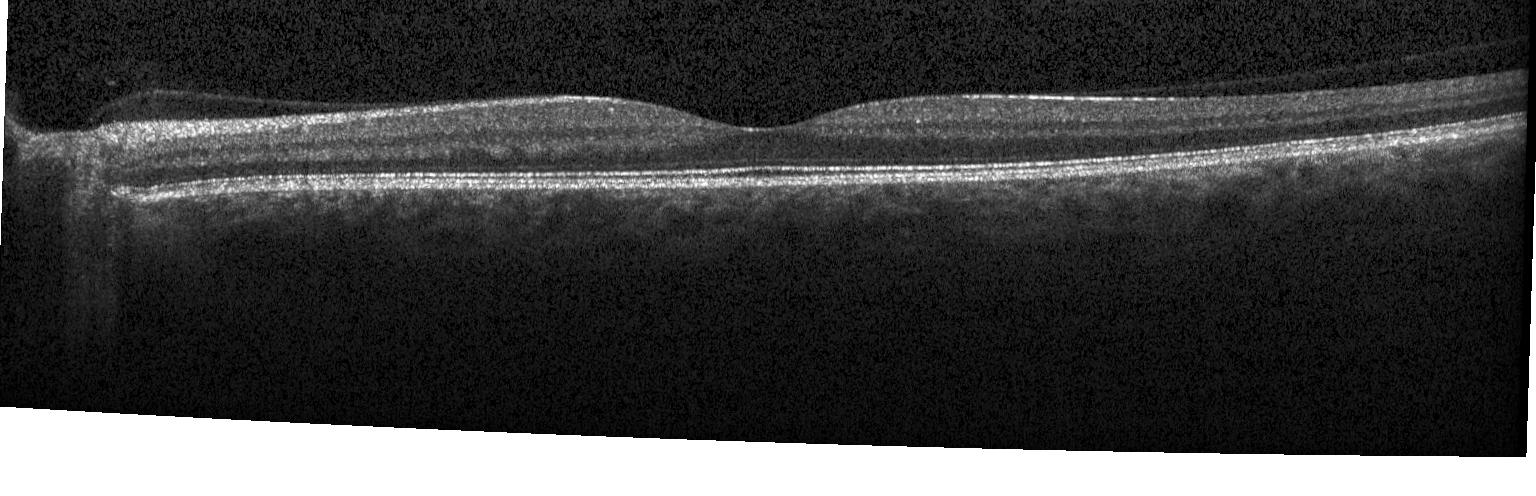

Finding: neither CNV, DME, nor drusen.